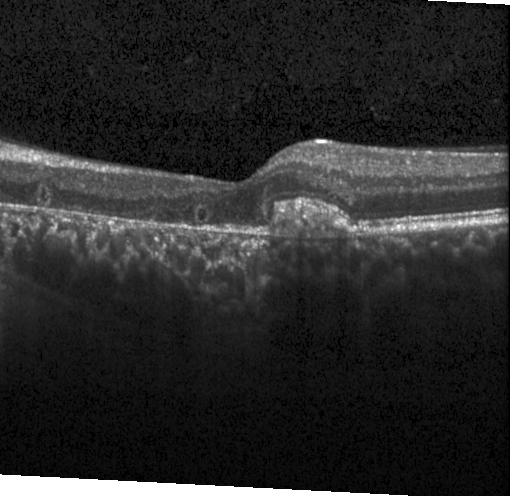
Instrument: Heidelberg Spectralis · optical coherence tomography scan · spectral-domain OCT
Dx: choroidal neovascularization (CNV).